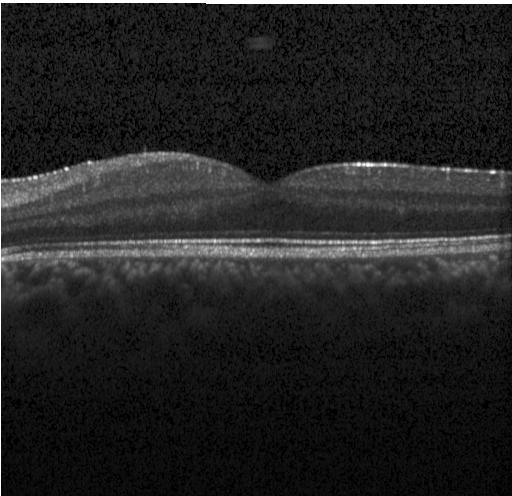

Fovea-centered, Heidelberg Spectralis, retinal OCT B-scan, spectral-domain optical coherence tomography.
This B-scan demonstrates no evidence of choroidal neovascularization, diabetic macular edema, or drusen.